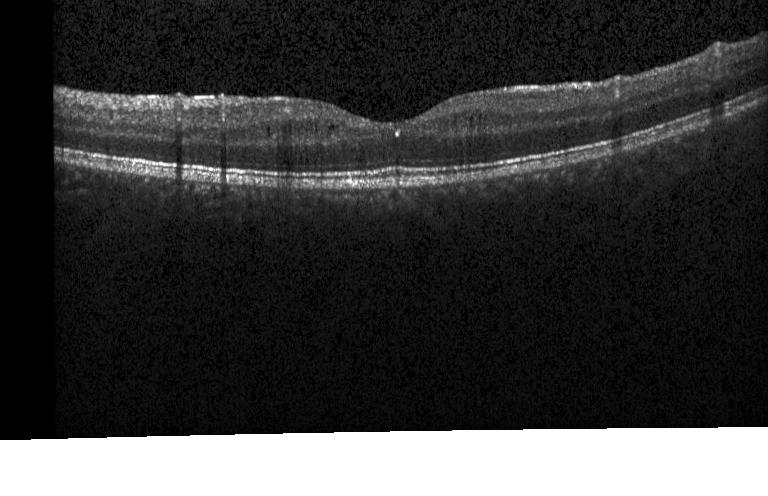 SD-OCT; optical coherence tomography B-scan; instrument: Heidelberg Spectralis. Diagnosis: diabetic macular edema.